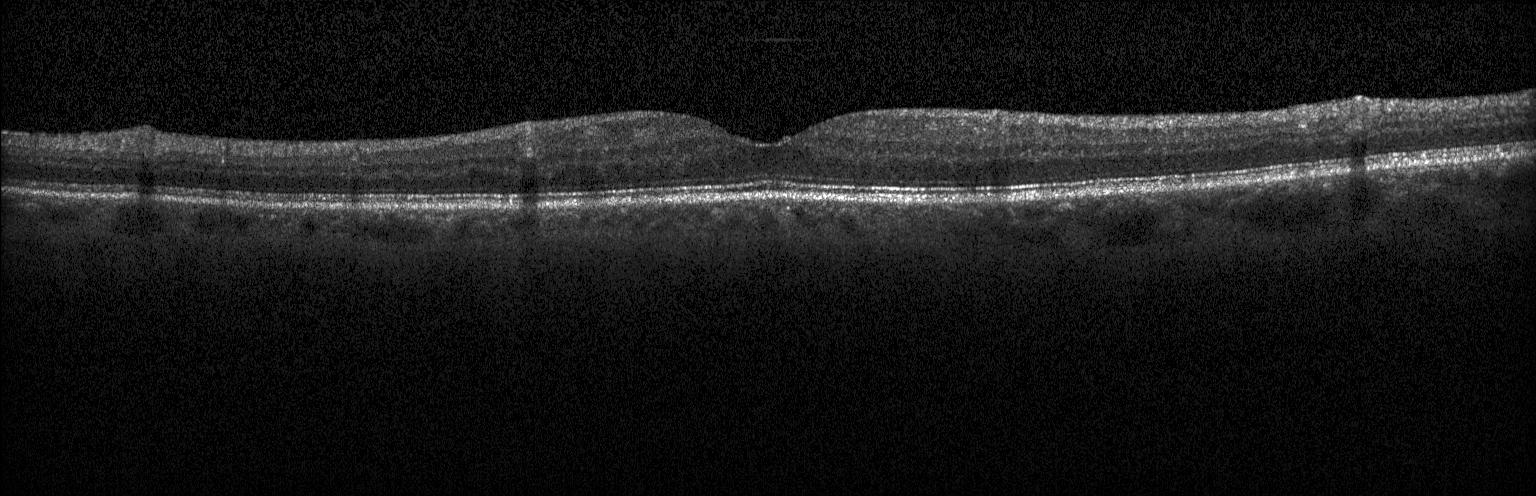
Finding: neither choroidal neovascularization, diabetic macular edema, nor drusen.